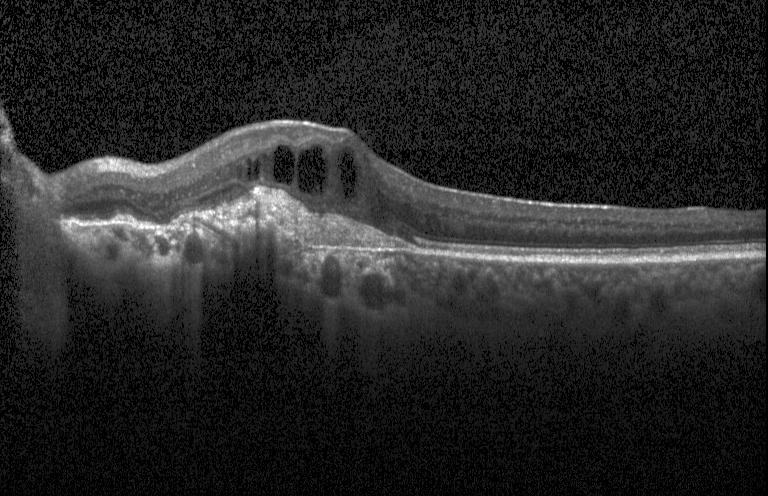 Spectral-domain OCT, optical coherence tomography B-scan, Heidelberg Spectralis OCT system, fovea-centered
Impression: a choroidal neovascular membrane.